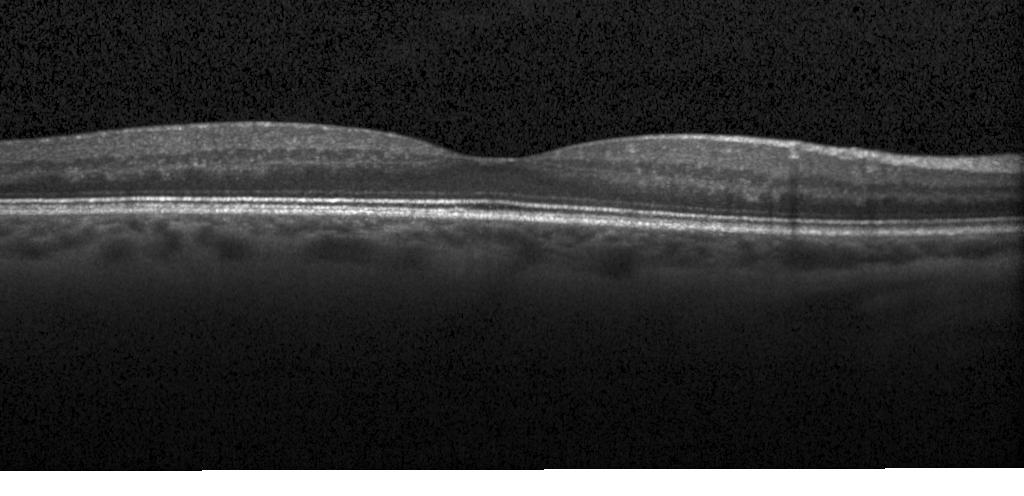

Optical coherence tomography B-scan; Heidelberg Spectralis; centered on the fovea.
The scan shows no CNV, DME, or drusen.